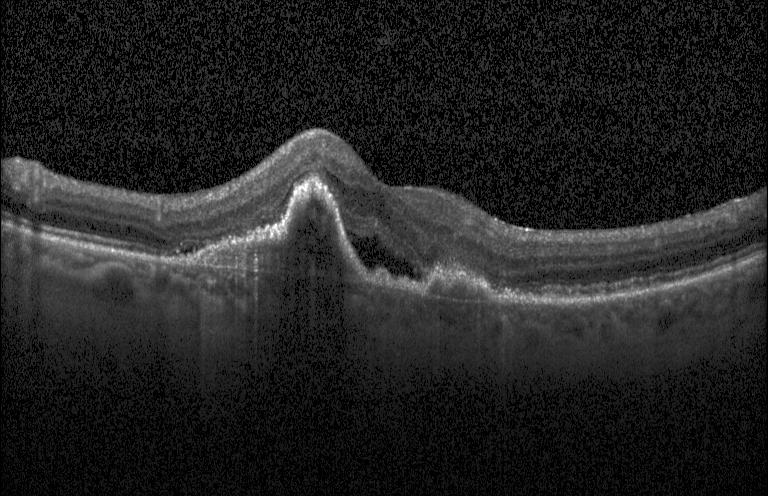

Dx: a choroidal neovascular membrane.